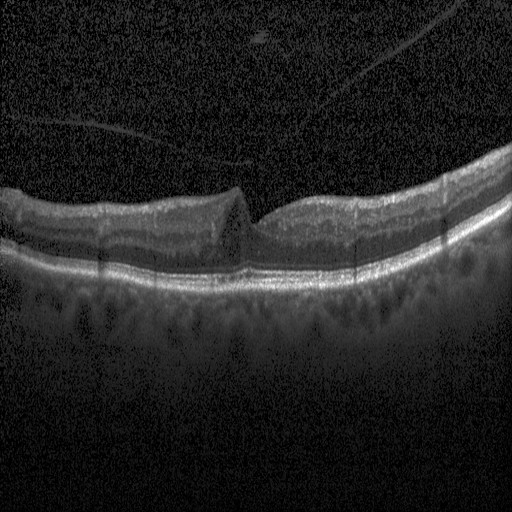

This B-scan demonstrates DME.